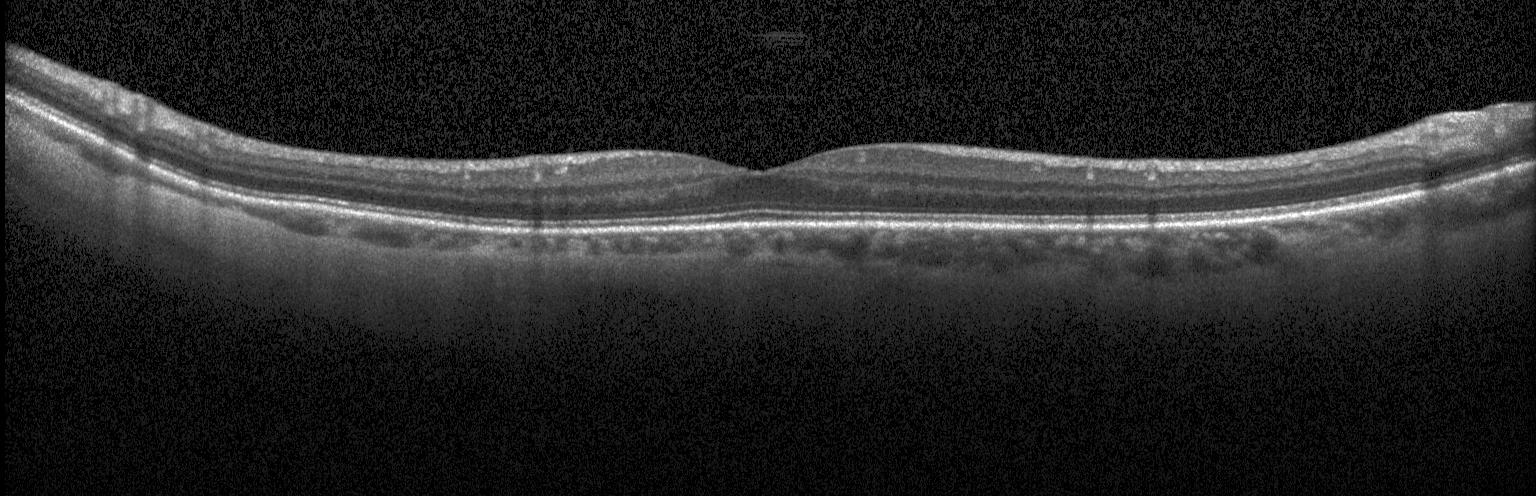 Centered on the fovea. Heidelberg Spectralis OCT system. Optical coherence tomography B-scan. SD-OCT — Impression: neither choroidal neovascularization, diabetic macular edema, nor drusen.